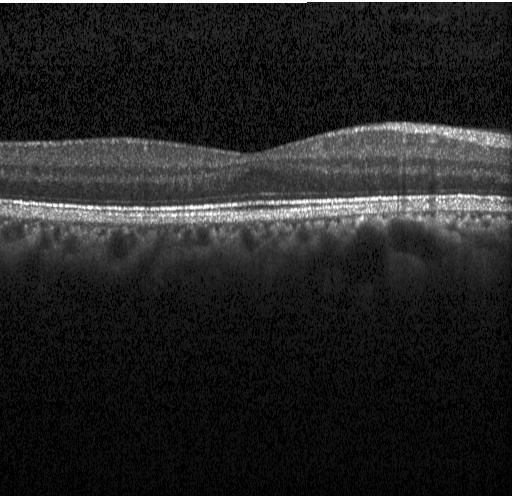 Optical coherence tomography B-scan · SD-OCT.
Impression: no choroidal neovascularization, no diabetic macular edema, and no drusen.